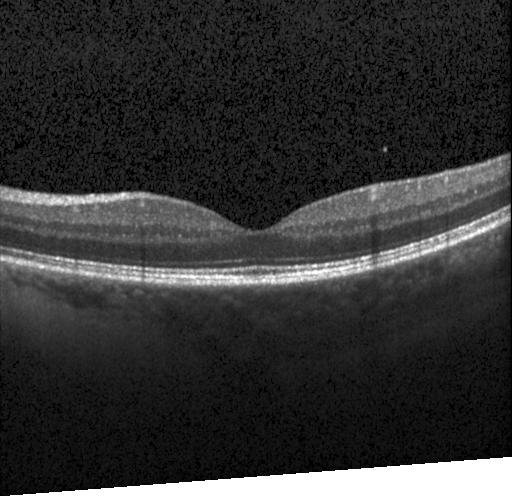

Spectral-domain OCT. Optical coherence tomography scan.
Assessment: no evidence of choroidal neovascularization, diabetic macular edema, or drusen.